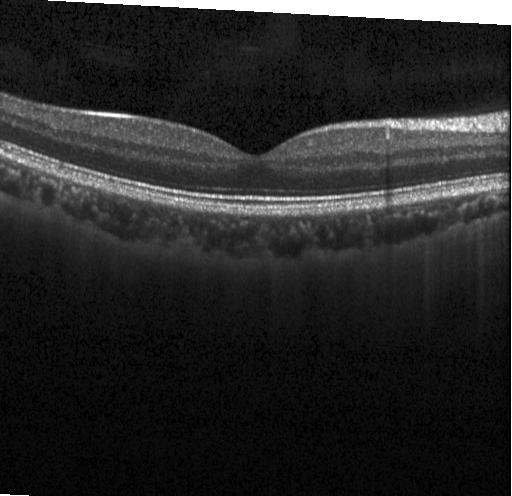 SD-OCT; retinal OCT cross-section — Impression: no choroidal neovascularization, no diabetic macular edema, and no drusen.